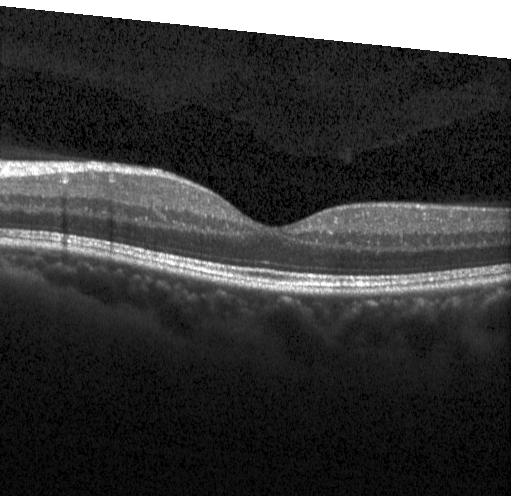

Through the macula. Heidelberg Spectralis OCT system. Retinal OCT cross-section — Assessment: neither choroidal neovascularization, diabetic macular edema, nor drusen.